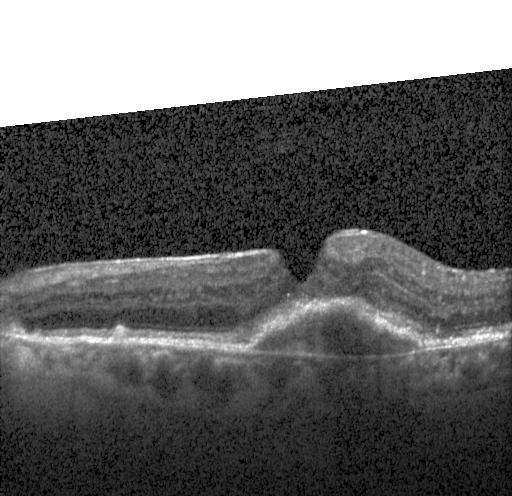 OCT B-scan
Finding: choroidal neovascularization.